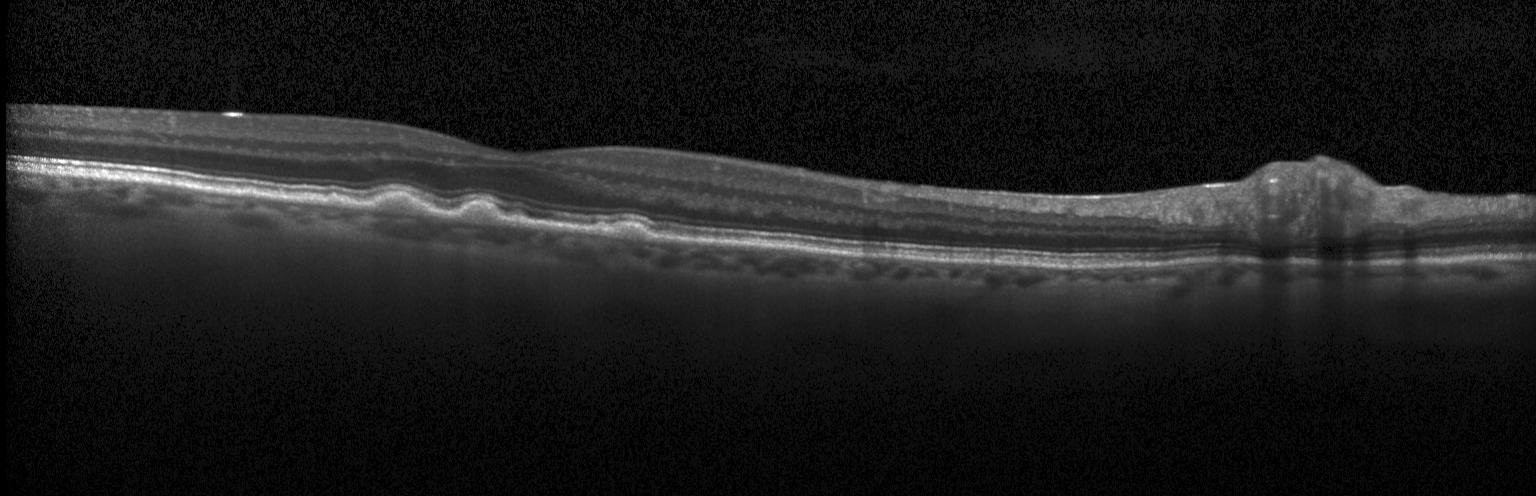
OCT B-scan.
Dx: sub-RPE drusenoid deposits.